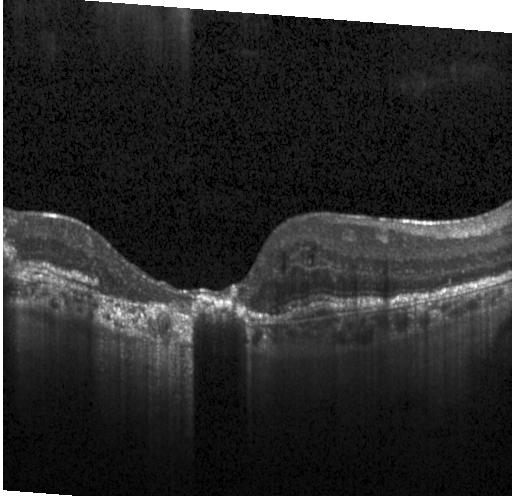
A choroidal neovascular membrane.